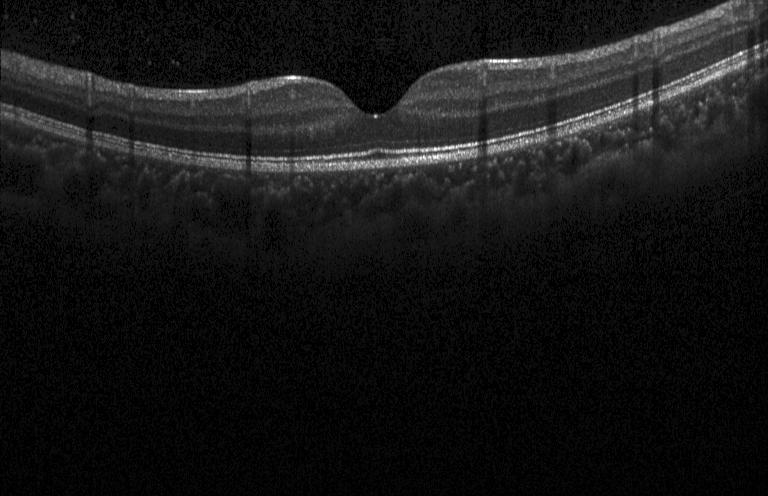

Centered on the fovea · spectral-domain optical coherence tomography · OCT B-scan — Dx: no evidence of CNV, DME, or drusen.